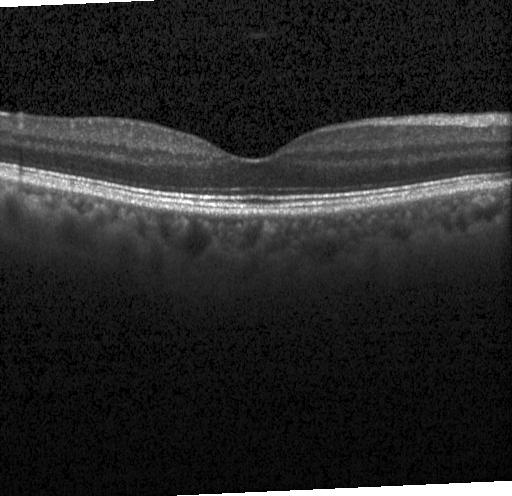 Spectral-domain OCT. Acquired on a Heidelberg Spectralis. OCT line scan. Horizontal scan through the fovea
Finding: no evidence of choroidal neovascularization, diabetic macular edema, or drusen.